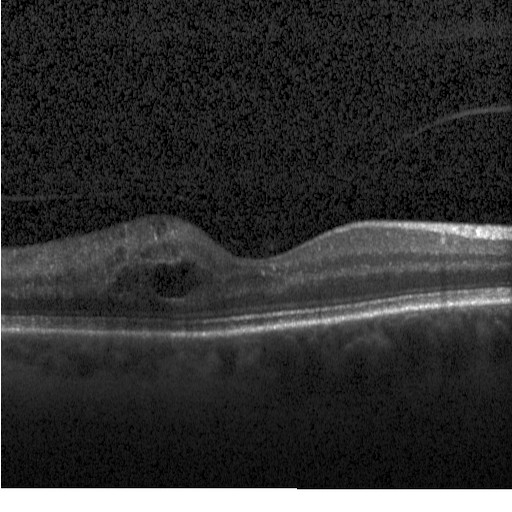 Impression: DME.